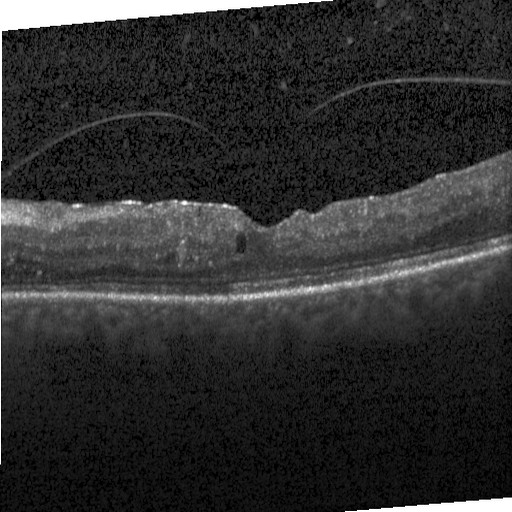

OCT B-scan.
Diagnosis: DME.